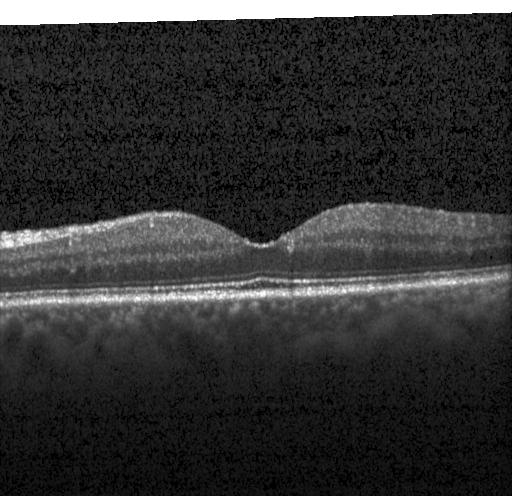
OCT line scan, SD-OCT. Dx: no choroidal neovascularization, diabetic macular edema, or drusen.